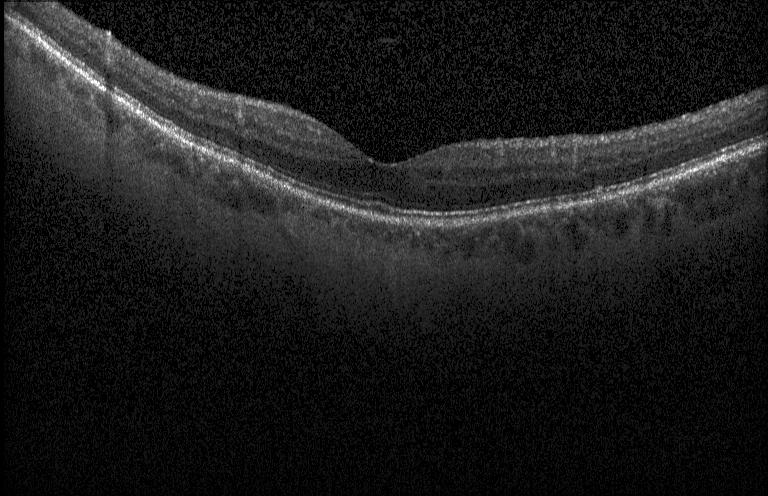

No evidence of choroidal neovascularization, diabetic macular edema, or drusen.